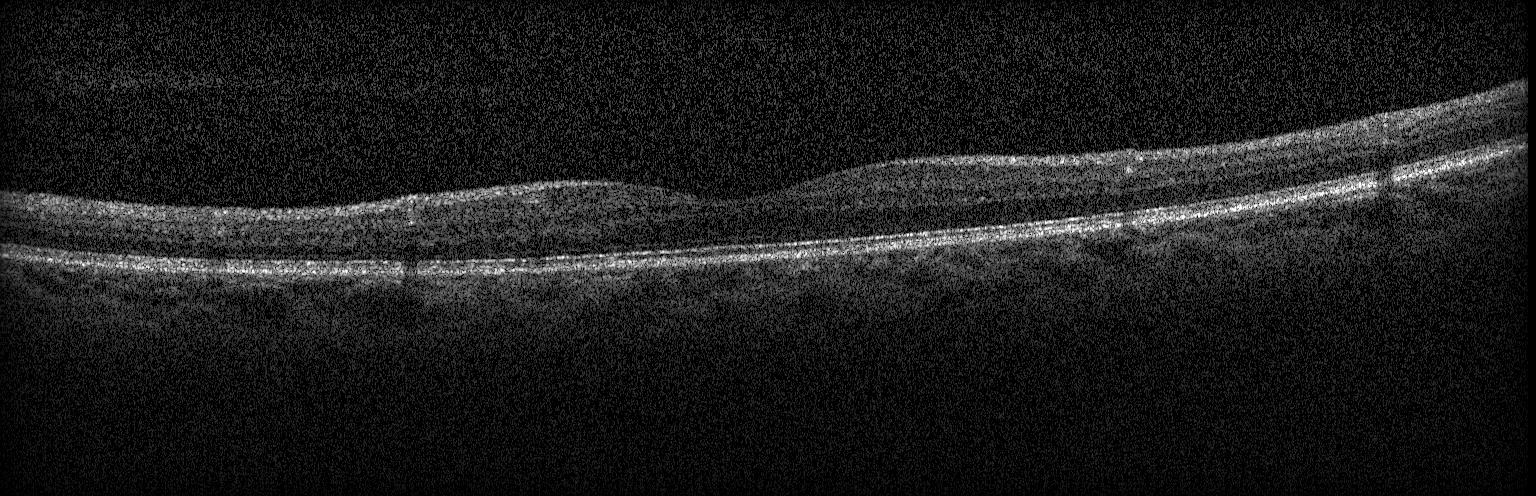

SD-OCT, optical coherence tomography B-scan, centered on the fovea.
This B-scan demonstrates no choroidal neovascularization, diabetic macular edema, or drusen.